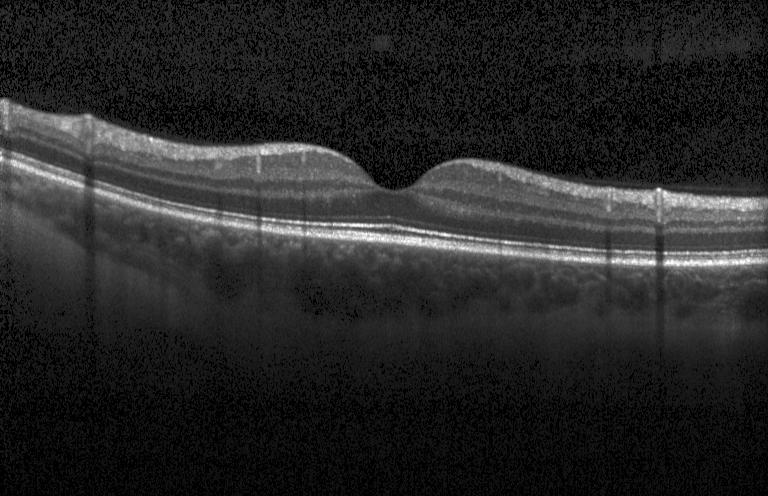
OCT line scan. Impression: no evidence of CNV, DME, or drusen.